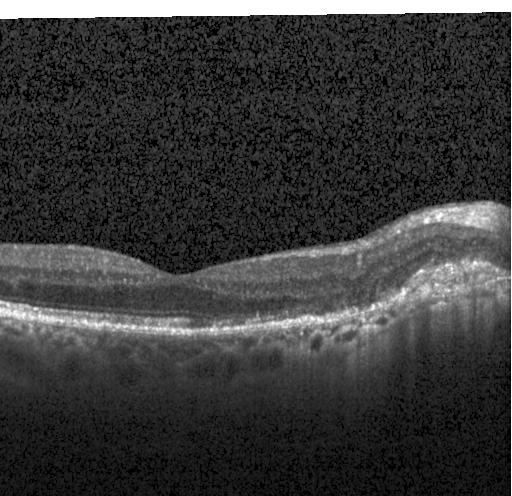 Retinal OCT B-scan, macular scan, spectral-domain OCT. Assessment: choroidal neovascularization (CNV).